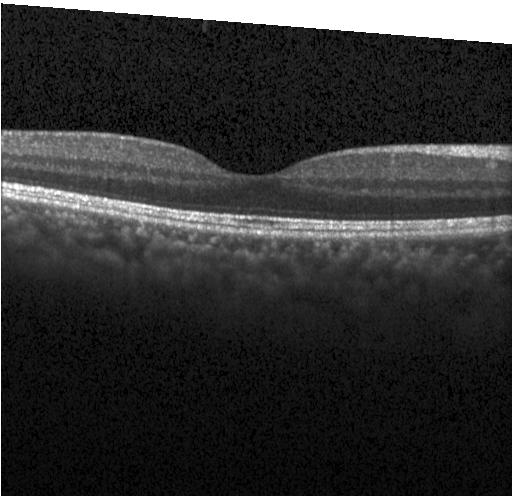 OCT finding: no choroidal neovascularization, diabetic macular edema, or drusen.